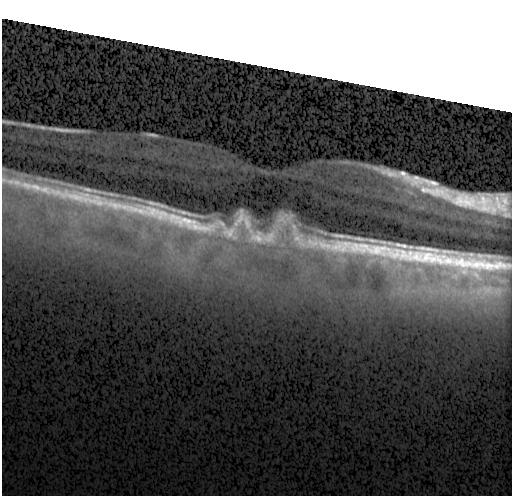
Retinal OCT B-scan. This B-scan demonstrates drusen.